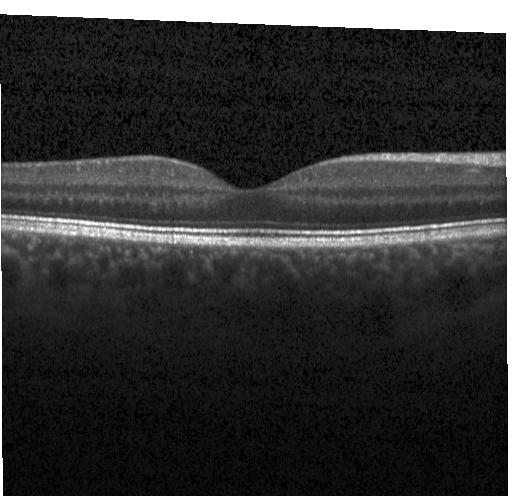 OCT B-scan
Impression: no choroidal neovascularization, diabetic macular edema, or drusen.